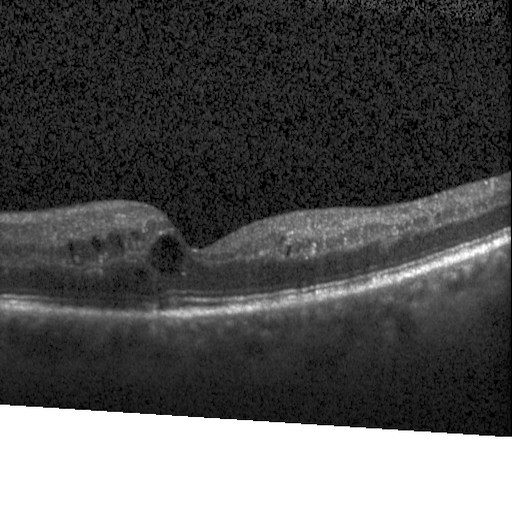 Instrument: Heidelberg Spectralis · optical coherence tomography scan. Diagnosis: DME.